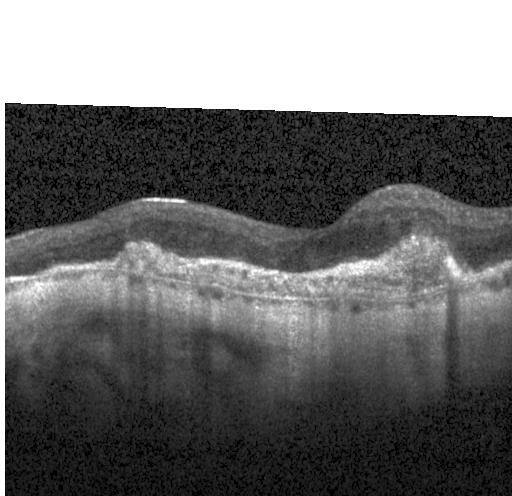
Retinal OCT cross-section; SD-OCT; Heidelberg Spectralis
Diagnosis: a choroidal neovascular membrane.